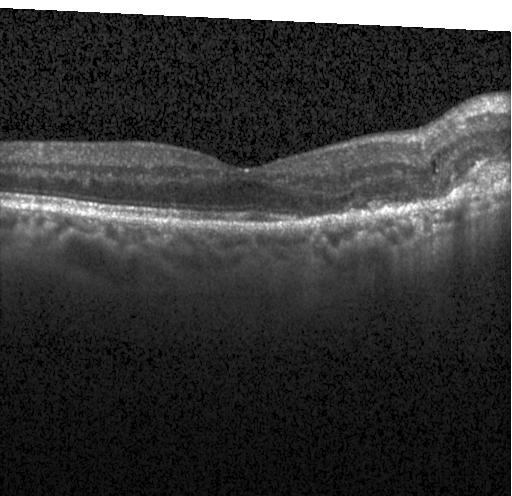

Impression: choroidal neovascularization (CNV).